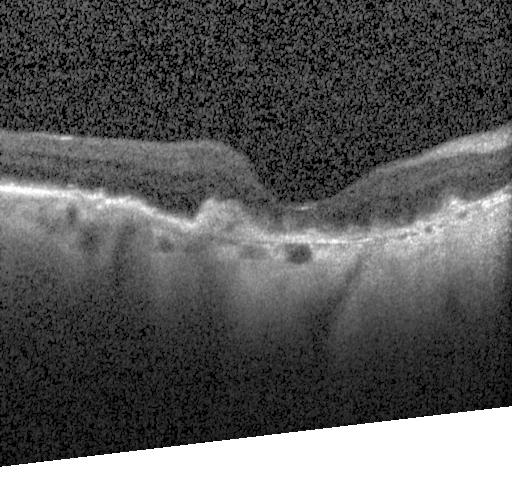 Heidelberg Spectralis · optical coherence tomography B-scan — Diagnosis: CNV.